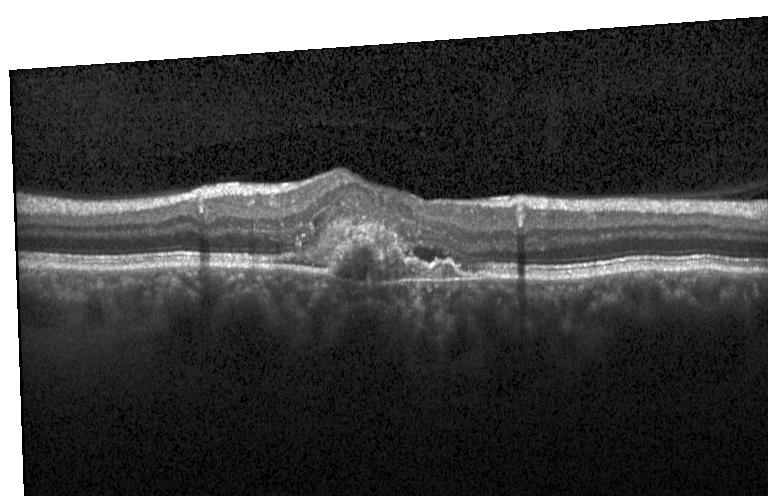
Finding: a choroidal neovascular membrane.